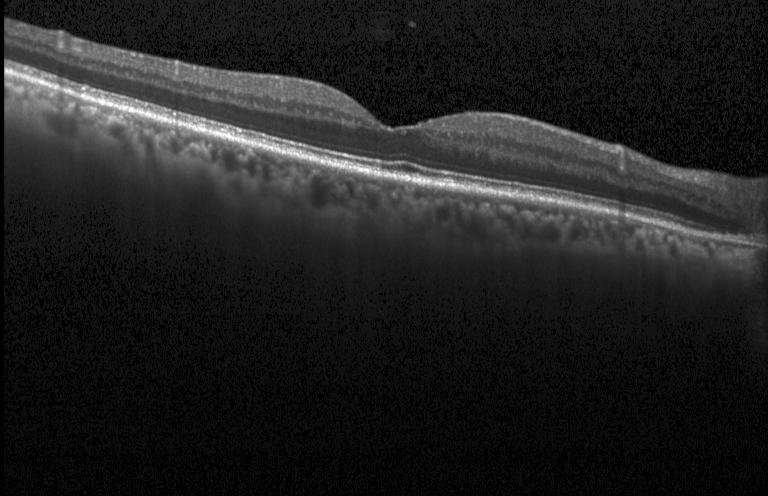
Horizontal scan through the fovea. Heidelberg Spectralis. Spectral-domain optical coherence tomography. Optical coherence tomography scan
Diagnosis: no choroidal neovascularization, diabetic macular edema, or drusen.